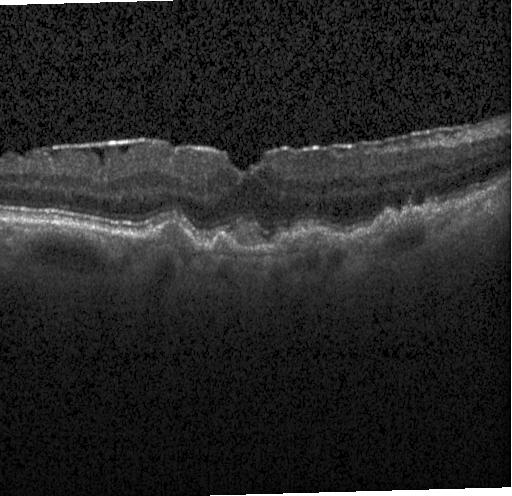
Heidelberg Spectralis, retinal OCT B-scan, SD-OCT, macular scan. Multiple drusen.